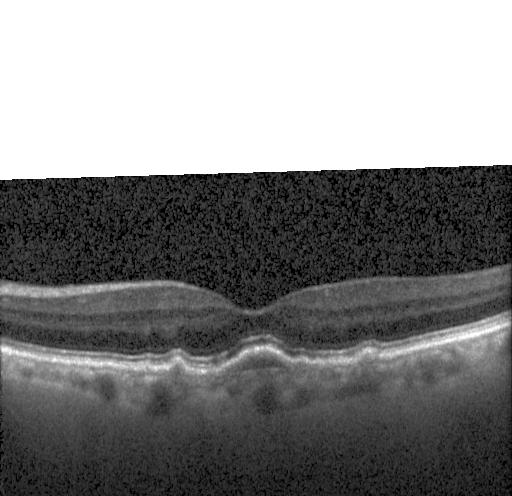

Impression: CNV.